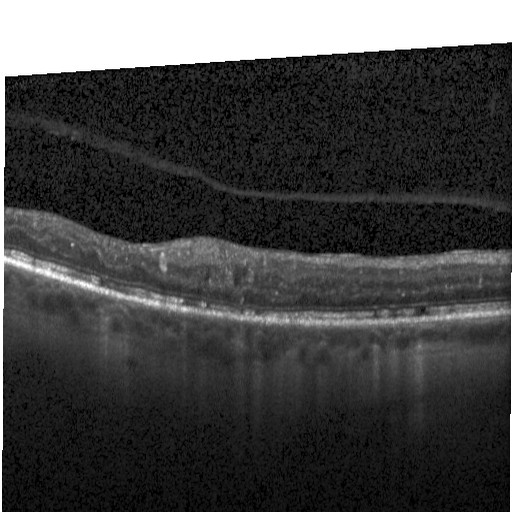 Finding: diabetic macular edema (DME).